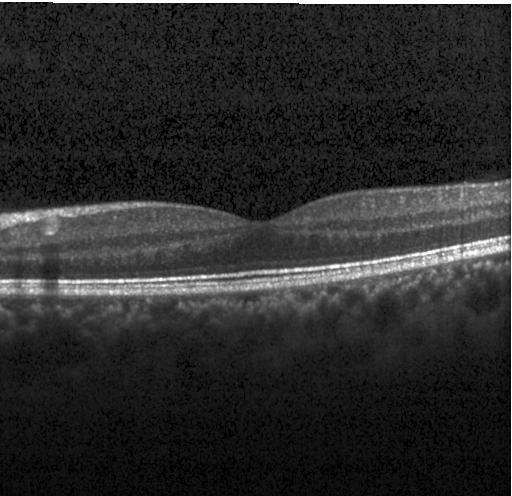 OCT line scan. Centered on the fovea. Acquired on a Heidelberg Spectralis. Spectral-domain optical coherence tomography — The scan shows neither CNV, DME, nor drusen.